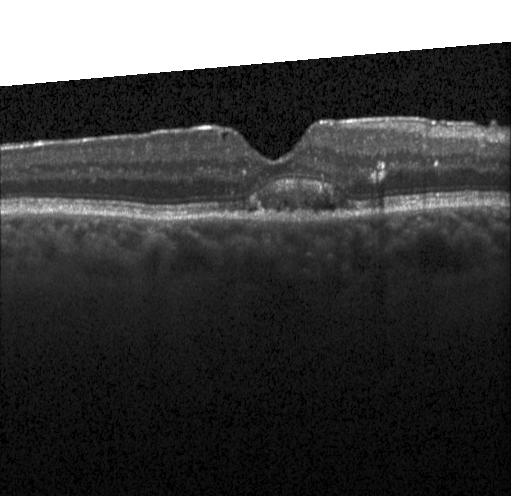
Retinal OCT cross-section — OCT finding: a choroidal neovascular membrane.